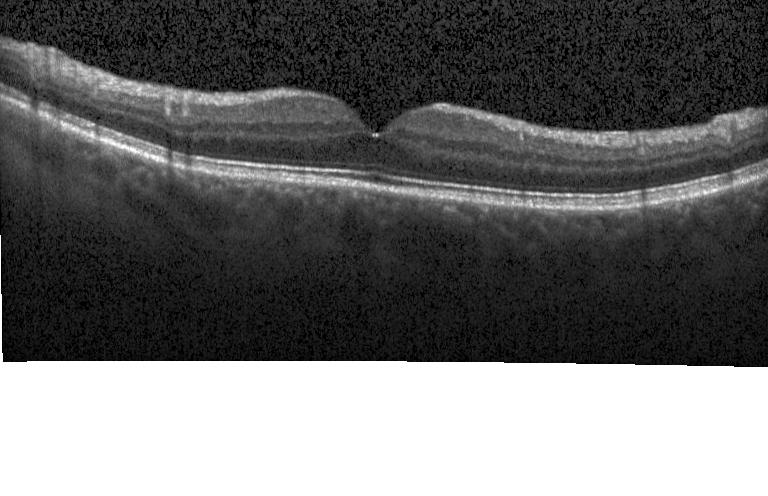 Instrument: Heidelberg Spectralis, SD-OCT, retinal OCT B-scan, through the macula.
Assessment: neither choroidal neovascularization, diabetic macular edema, nor drusen.